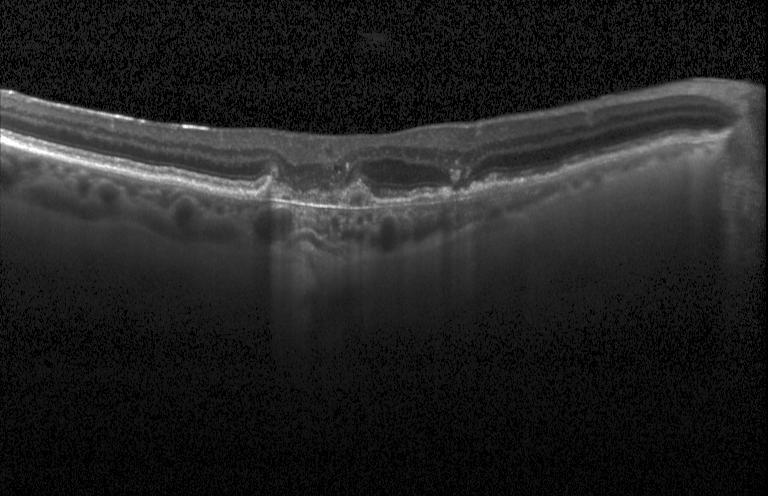 Instrument: Heidelberg Spectralis; retinal OCT B-scan
Diagnosis: choroidal neovascularization.